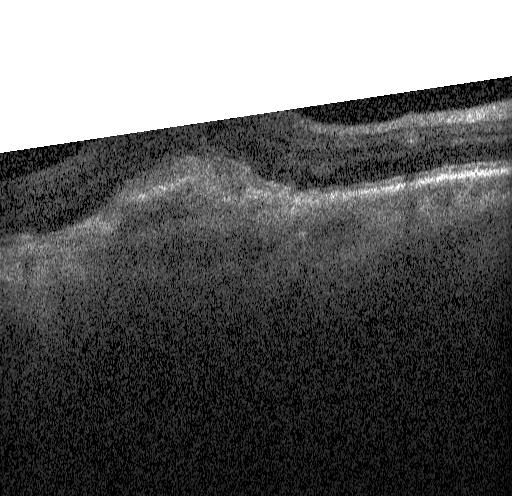
Instrument: Heidelberg Spectralis · retinal OCT B-scan. OCT finding: a choroidal neovascular membrane.